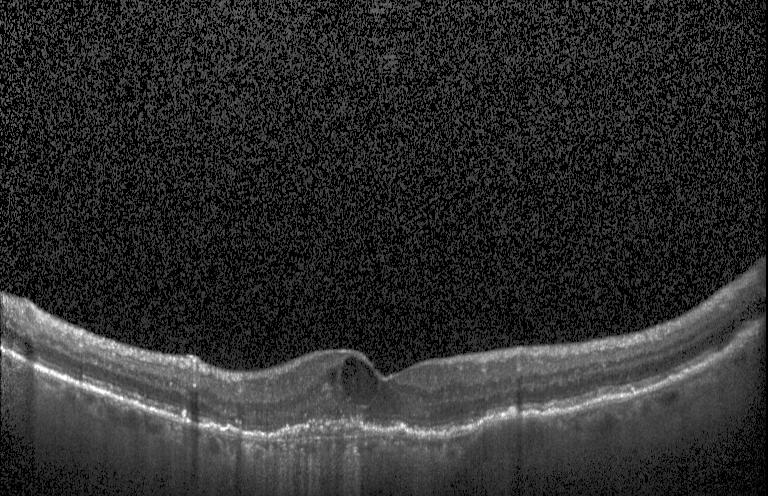

Impression: choroidal neovascularization.